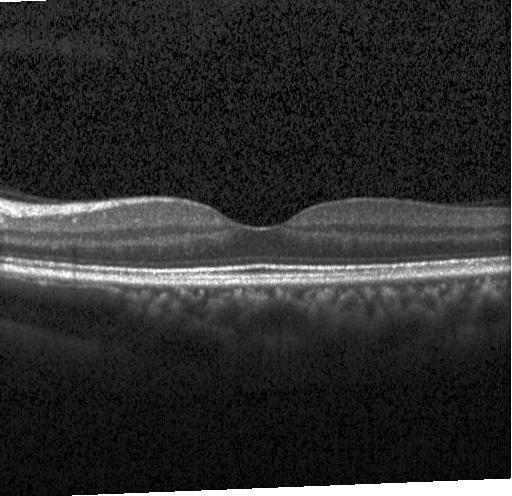 OCT B-scan; centered on the fovea. Diagnosis: no CNV, DME, or drusen.